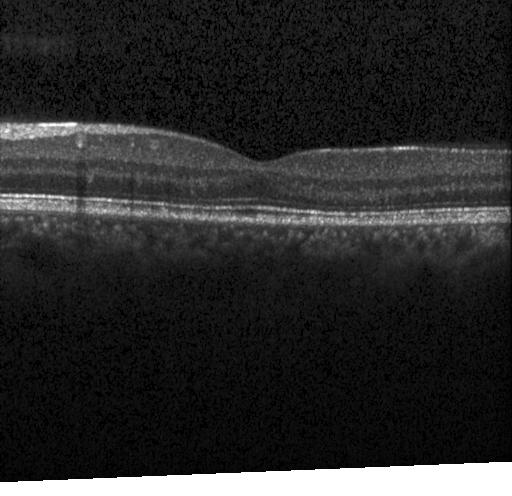
Instrument: Heidelberg Spectralis; centered on the fovea; retinal OCT cross-section.
Impression: no choroidal neovascularization, diabetic macular edema, or drusen.